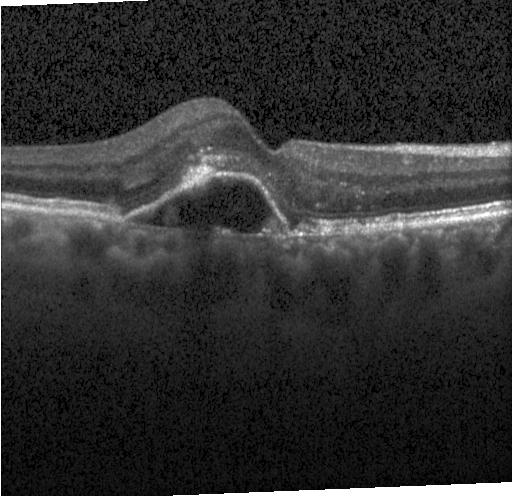

Impression: a choroidal neovascular membrane.